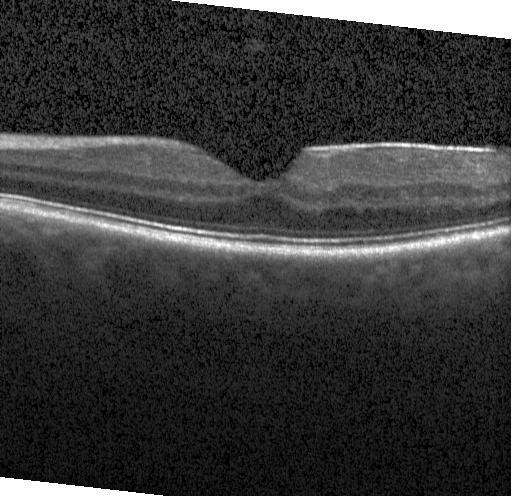

Horizontal scan through the fovea, OCT line scan — This B-scan demonstrates no choroidal neovascularization, diabetic macular edema, or drusen.